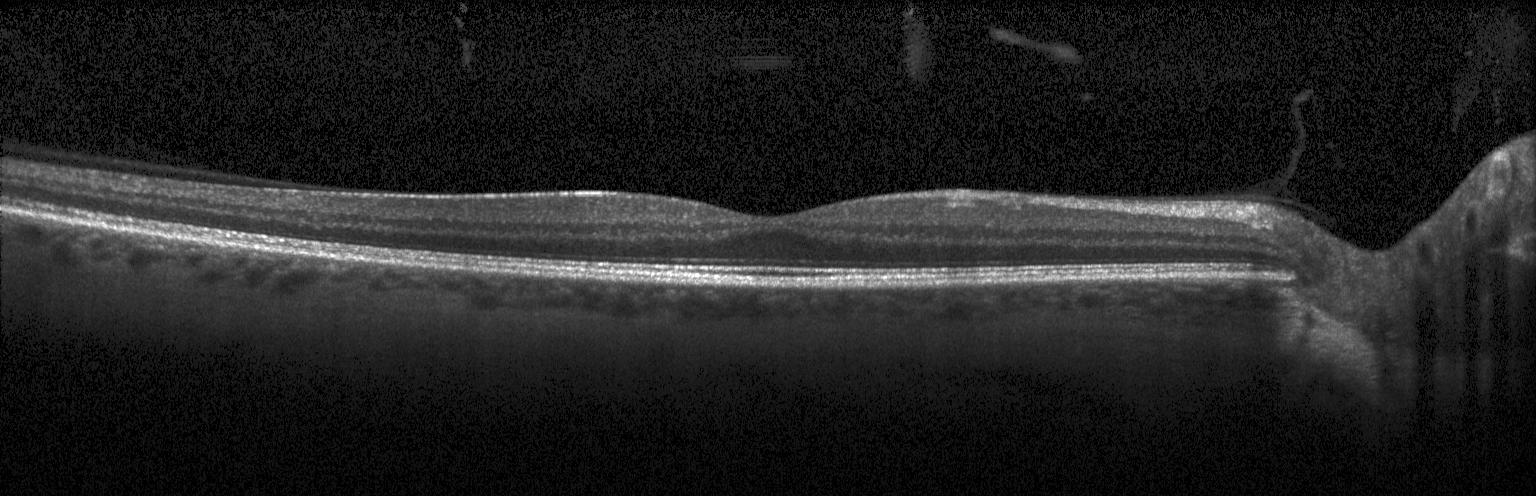

Optical coherence tomography scan, instrument: Heidelberg Spectralis, SD-OCT, horizontal scan through the fovea. Finding: no CNV, DME, or drusen.